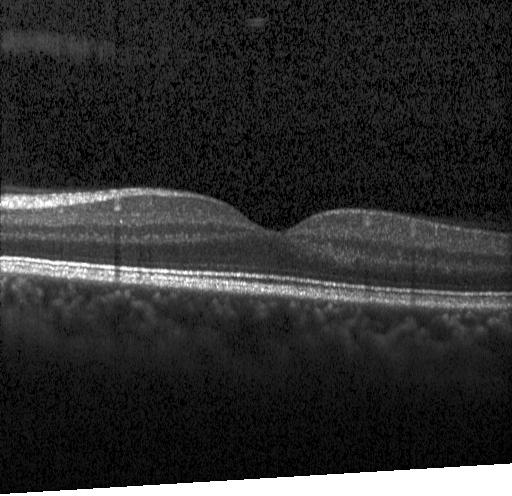 Diagnosis: no choroidal neovascularization, no diabetic macular edema, and no drusen.